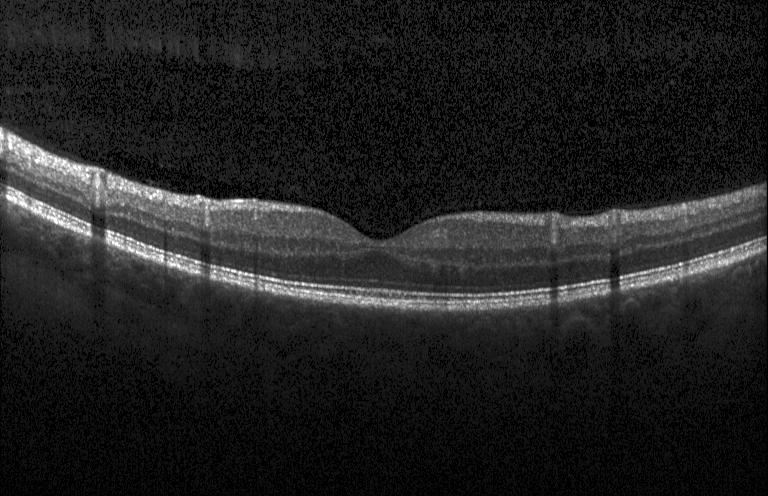

Dx: no choroidal neovascularization, diabetic macular edema, or drusen.